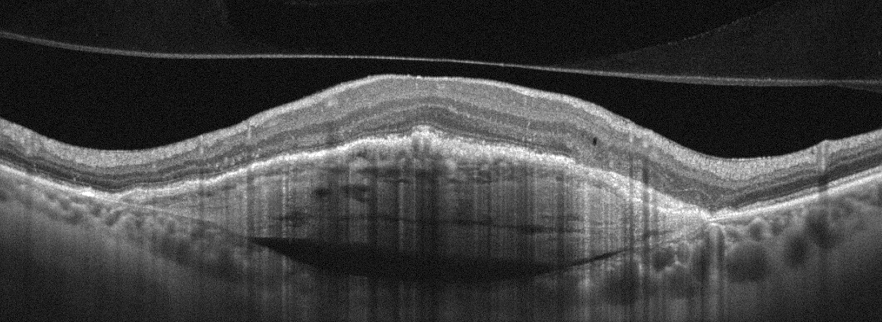
OCT B-scan, OD. Assessment: AMD.